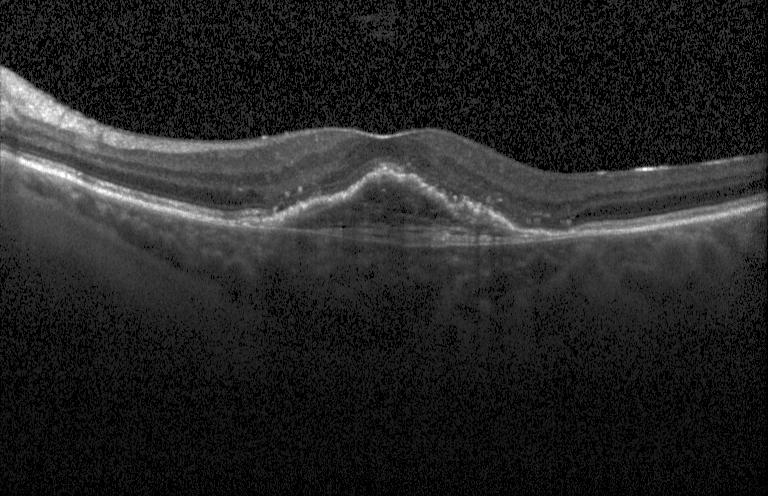 OCT B-scan — The scan shows a choroidal neovascular membrane.